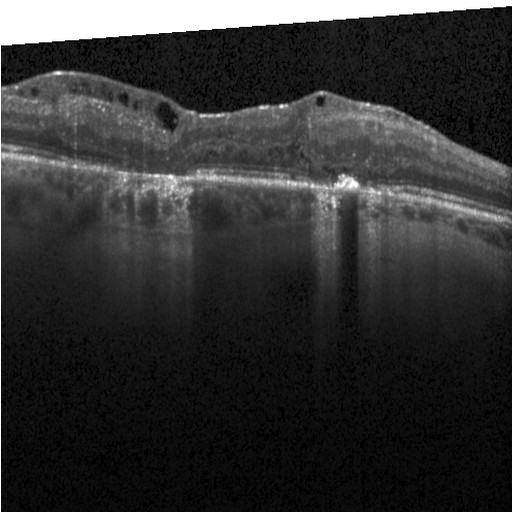 Diabetic macular edema.